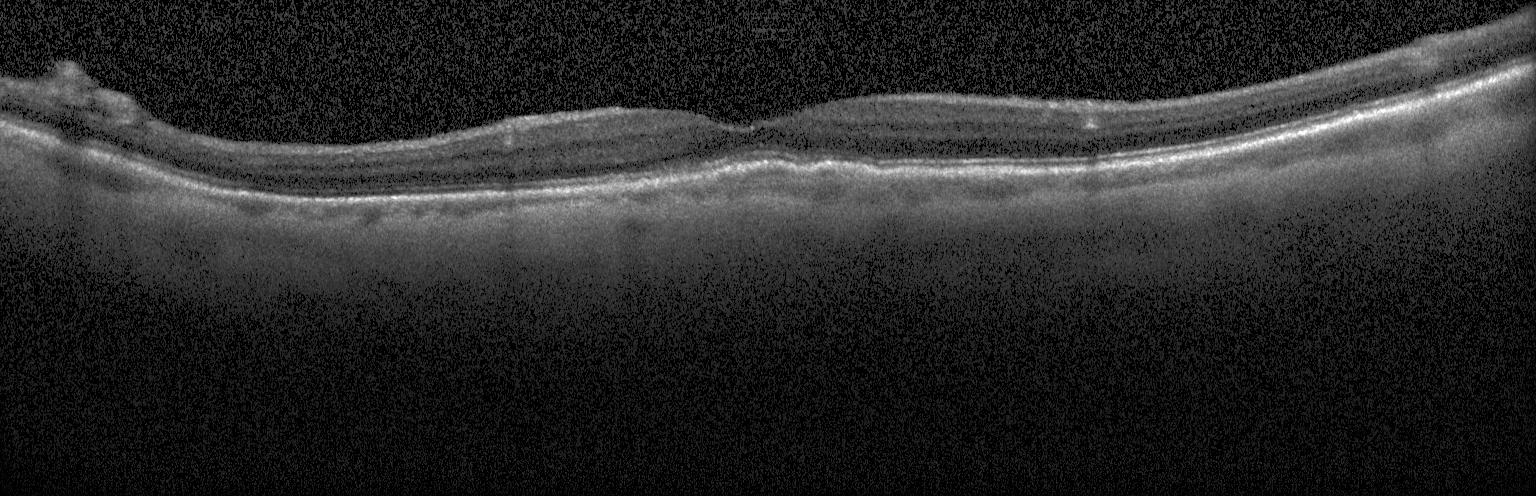 SD-OCT, through the macula, optical coherence tomography B-scan.
Finding: CNV.